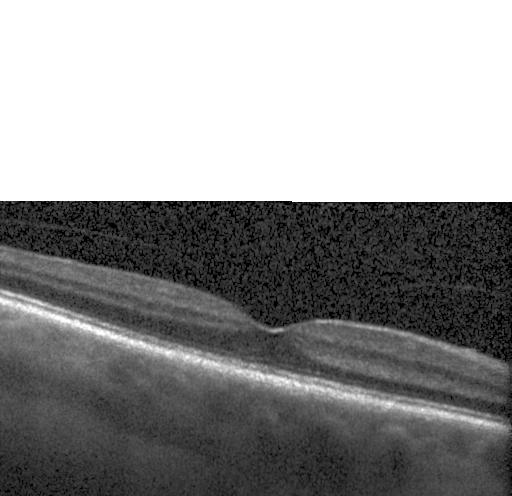 Finding: neither choroidal neovascularization, diabetic macular edema, nor drusen.